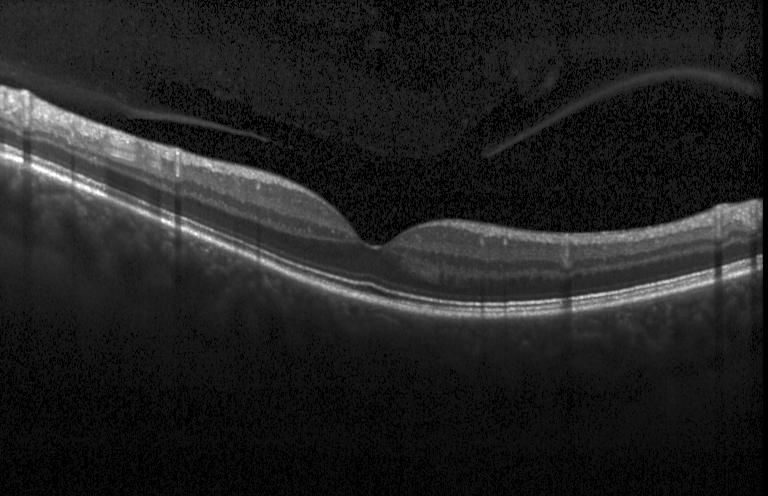
Spectral-domain OCT B-scan: no choroidal neovascularization, diabetic macular edema, or drusen.